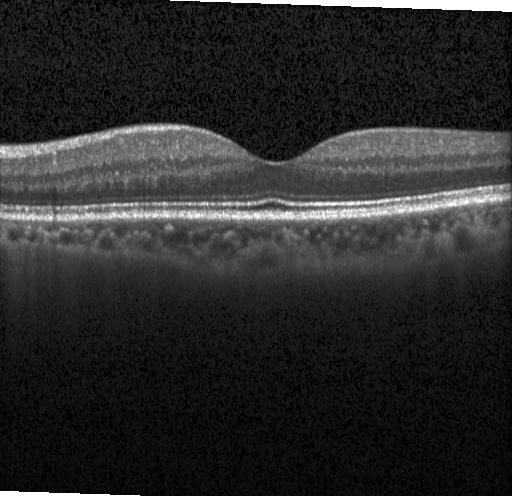 OCT B-scan showing no evidence of choroidal neovascularization, diabetic macular edema, or drusen.